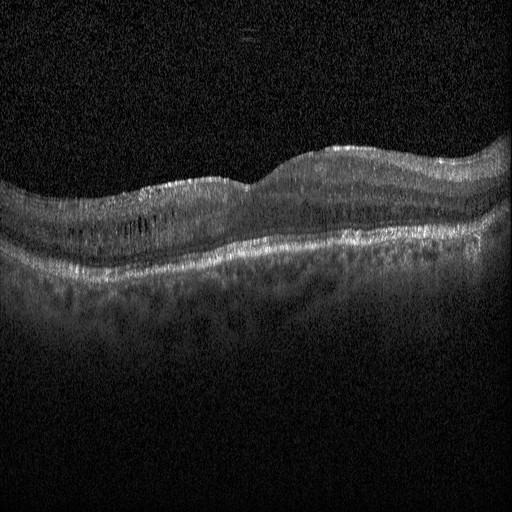
SD-OCT. Fovea-centered. Acquired on a Heidelberg Spectralis. Optical coherence tomography scan
The scan shows diabetic macular edema.